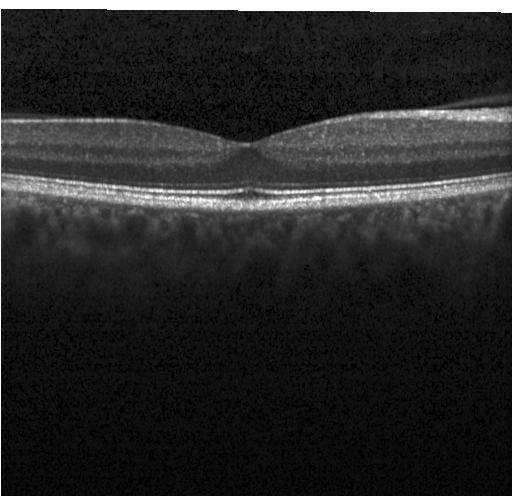
Retinal OCT cross-section — Impression: no choroidal neovascularization, no diabetic macular edema, and no drusen.